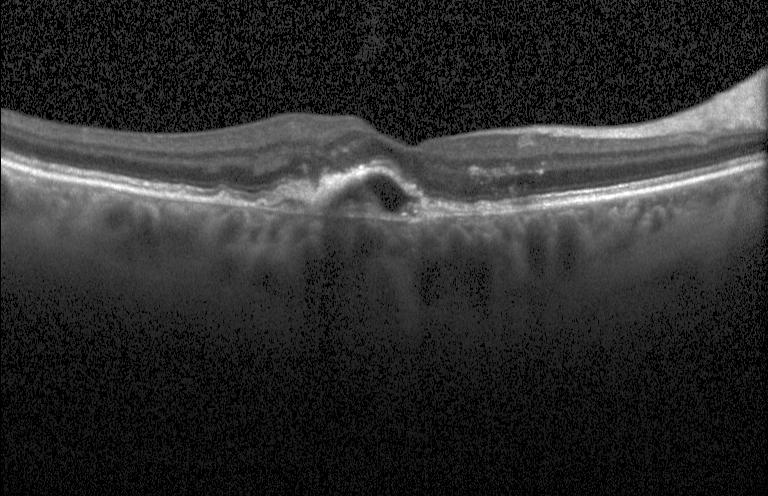

Retinal OCT cross-section showing a choroidal neovascular membrane.